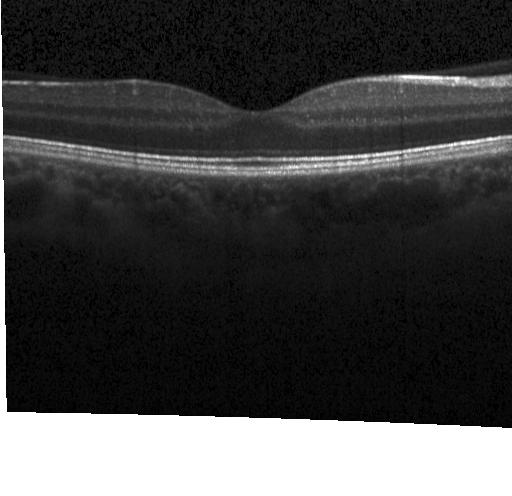
OCT B-scan
Diagnosis: no choroidal neovascularization, no diabetic macular edema, and no drusen.